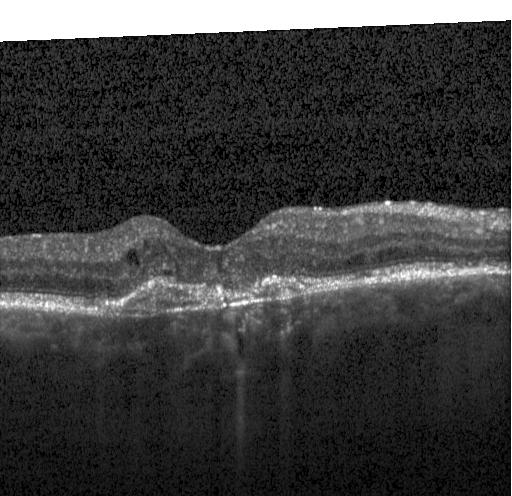
Spectral-domain OCT; macular scan; instrument: Heidelberg Spectralis; retinal OCT cross-section.
Assessment: a choroidal neovascular membrane.